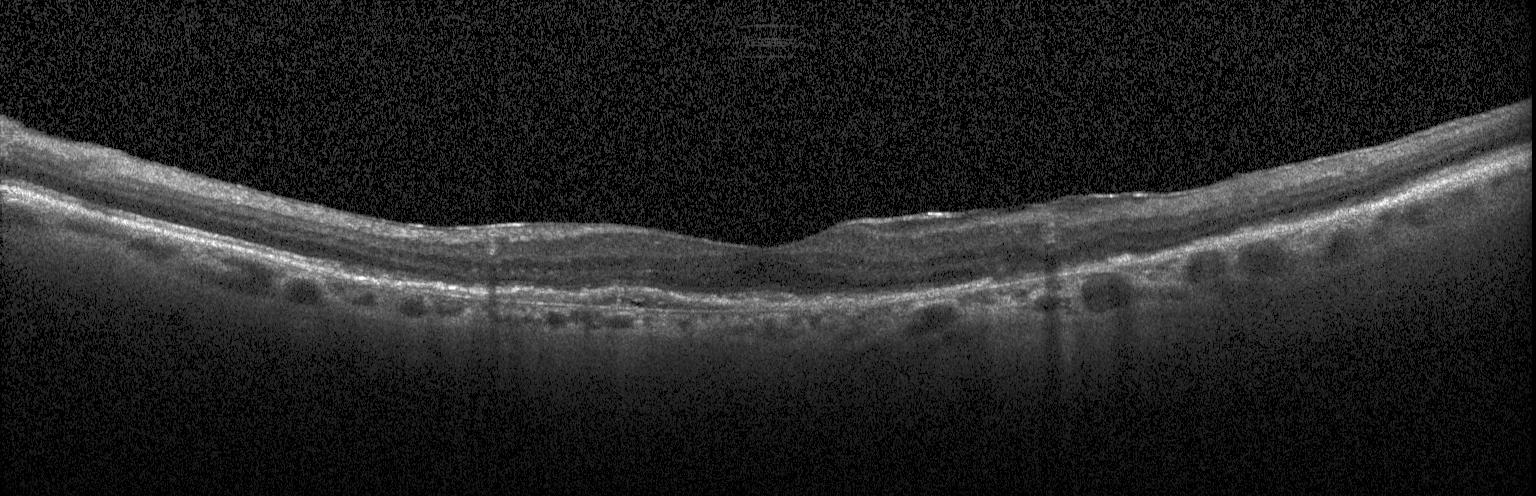
Optical coherence tomography B-scan — Finding: a choroidal neovascular membrane.